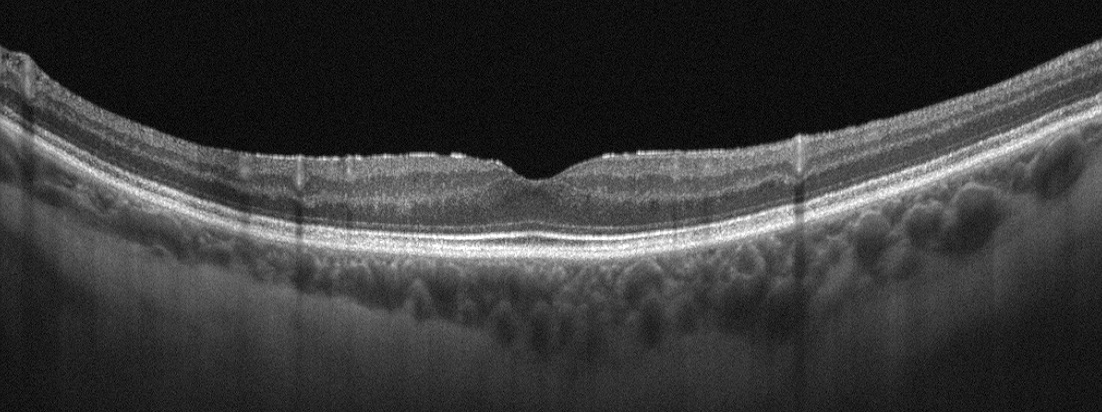 Retinal OCT B-scan, through the macula, instrument: Optovue Avanti RTVue XR — Impression: epiretinal membrane (ERM).